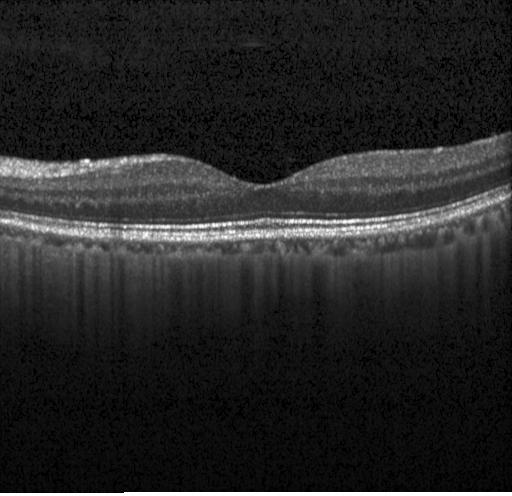

Instrument: Heidelberg Spectralis. Retinal OCT cross-section. Spectral-domain OCT.
Finding: no CNV, DME, or drusen.